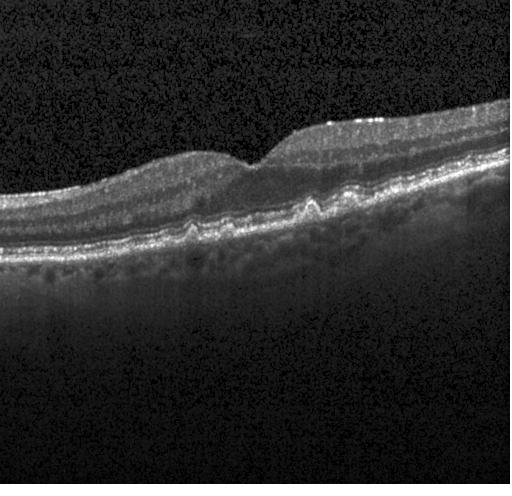
Fovea-centered · retinal OCT cross-section · acquired on a Heidelberg Spectralis. The scan shows multiple drusen.